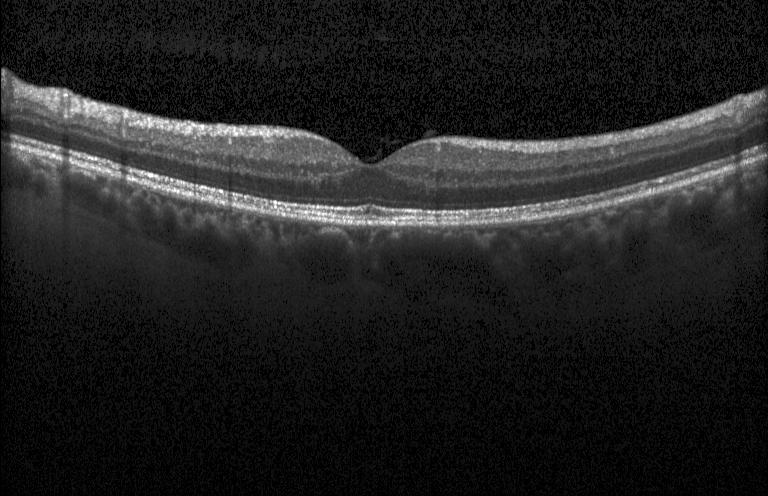
SD-OCT · OCT B-scan · through the macula.
The scan shows no choroidal neovascularization, no diabetic macular edema, and no drusen.